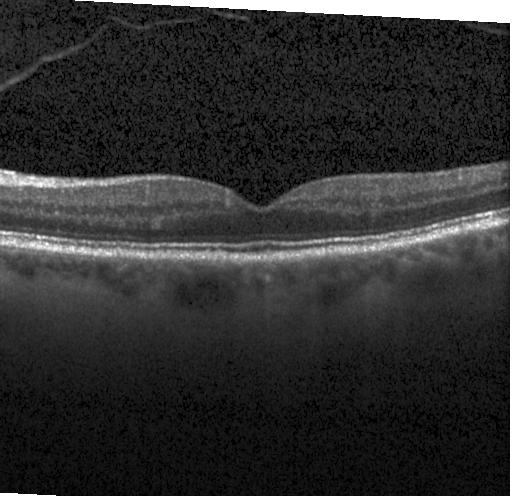

Diagnosis: no choroidal neovascularization, no diabetic macular edema, and no drusen.